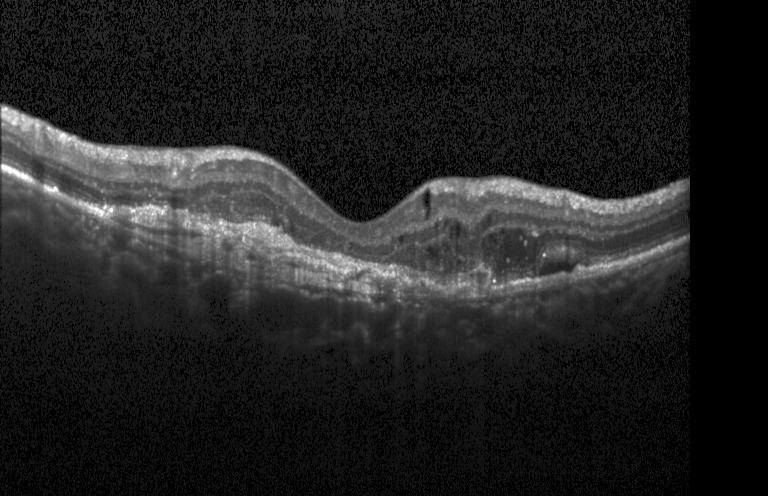

Retinal OCT cross-section. Acquired on a Heidelberg Spectralis. Impression: choroidal neovascularization.